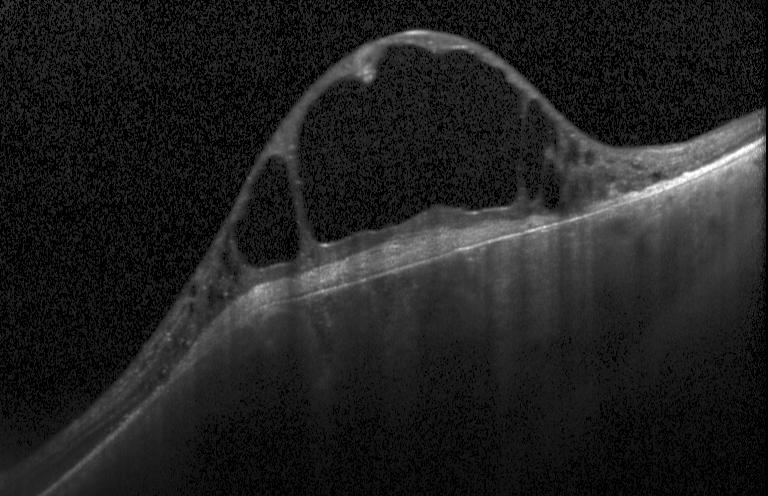
OCT B-scan — Impression: CNV.